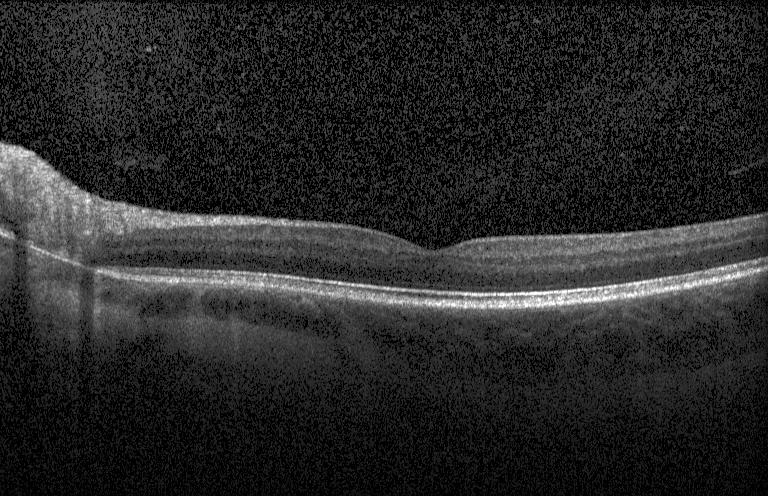 Dx: no CNV, DME, or drusen.